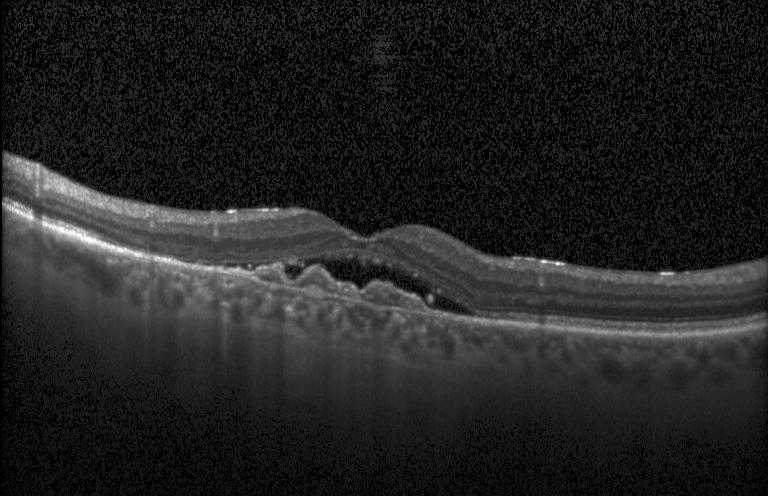

OCT scan showing choroidal neovascularization (CNV).